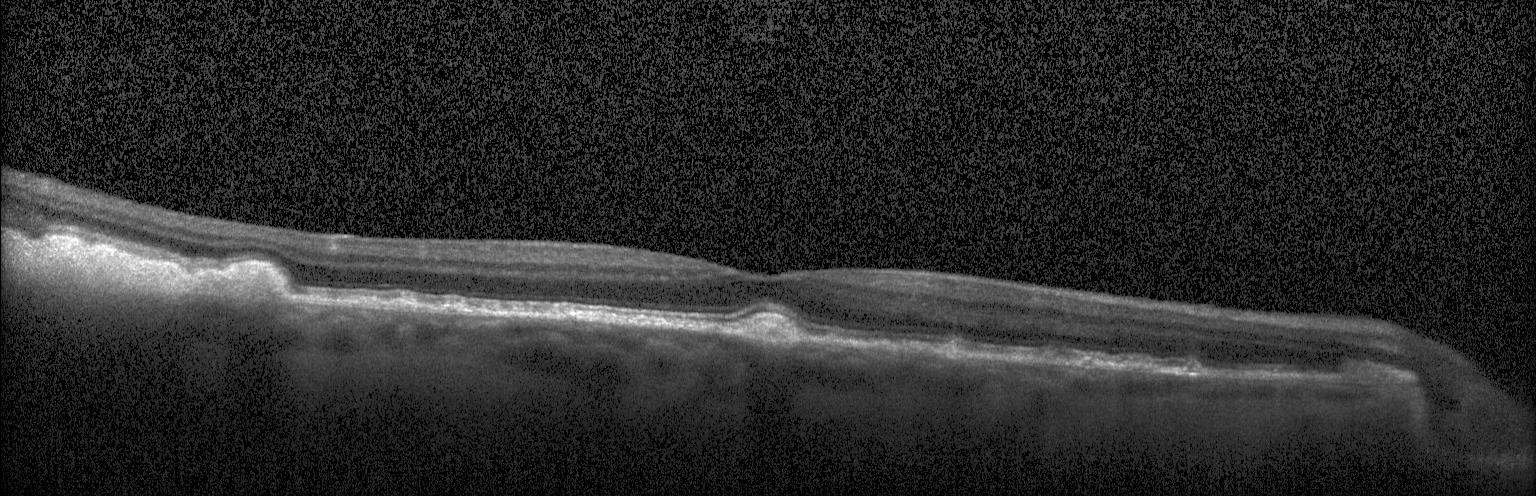

Retinal OCT cross-section showing drusen.